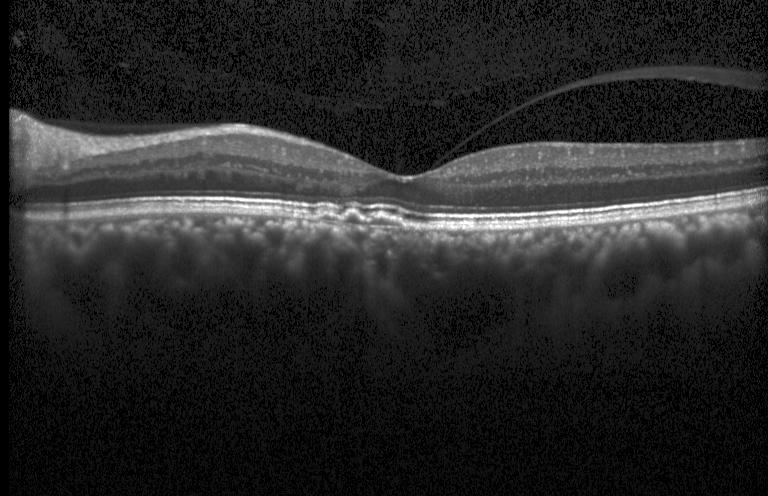
Instrument: Heidelberg Spectralis · retinal OCT B-scan · through the macula · spectral-domain OCT — Diagnosis: sub-RPE drusenoid deposits.